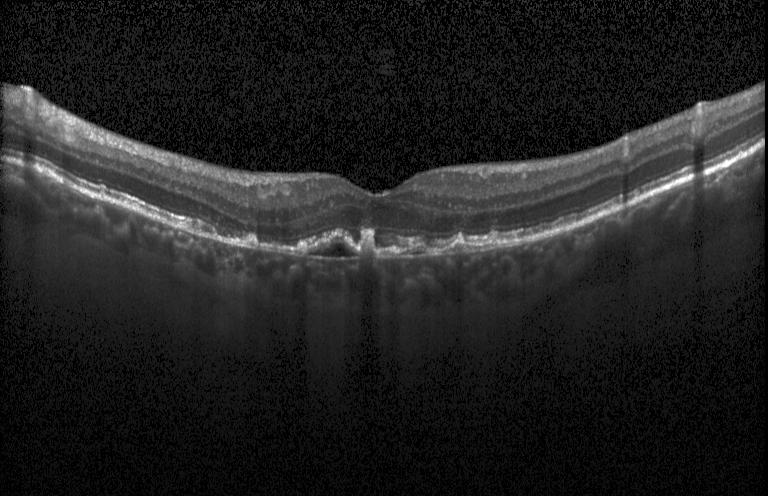 This B-scan demonstrates choroidal neovascularization.